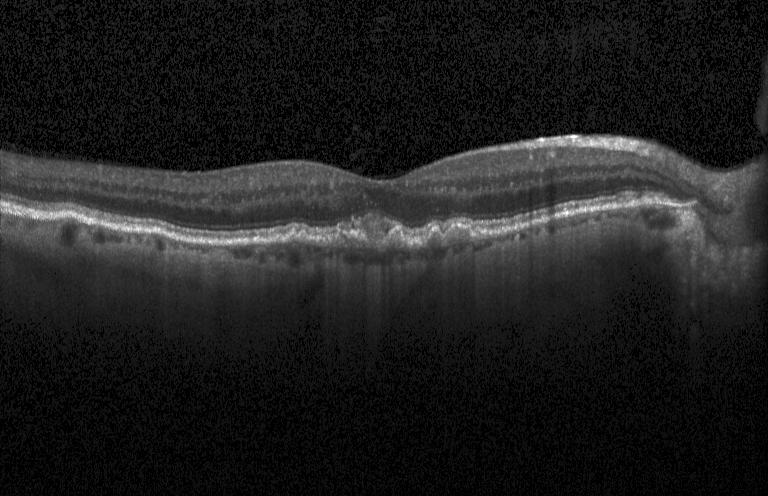
Diagnosis: multiple drusen.